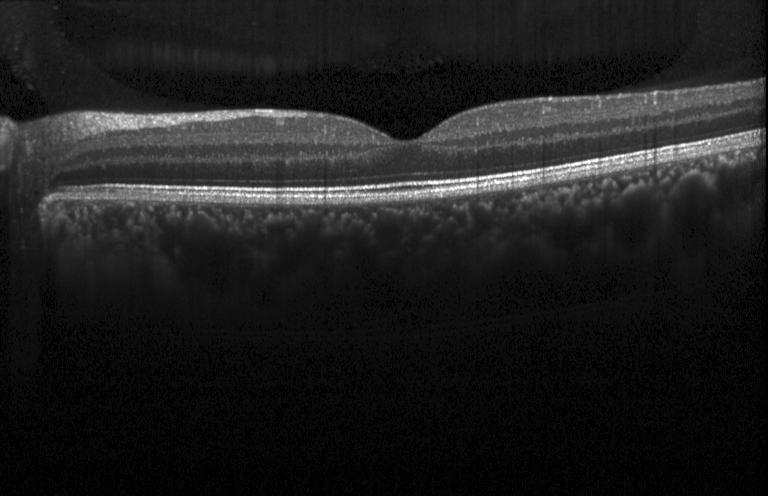 Fovea-centered. OCT line scan. SD-OCT — Dx: neither CNV, DME, nor drusen.